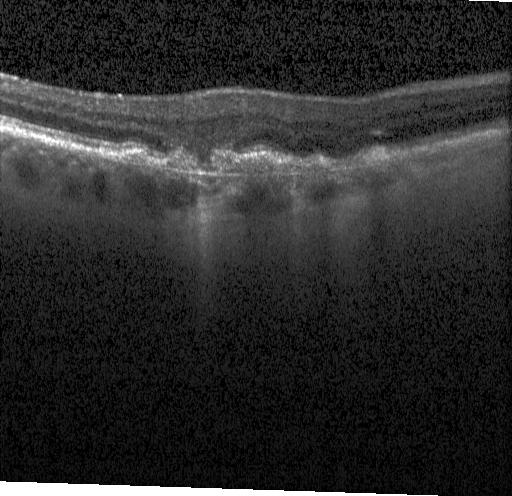

Assessment: CNV.